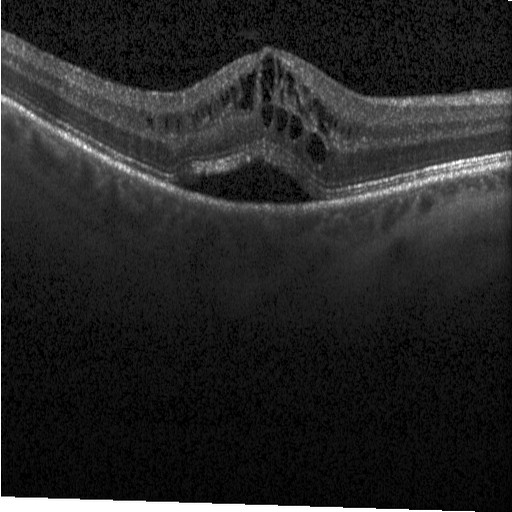

Diagnosis: diabetic macular edema (DME).